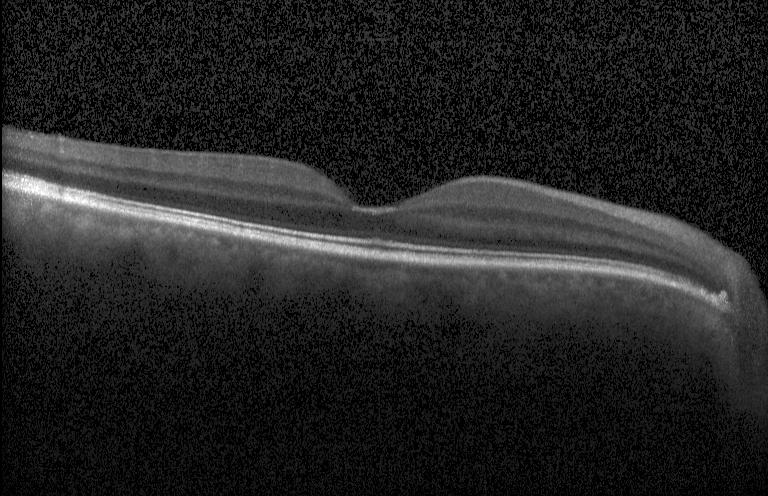

Macular OCT: neither choroidal neovascularization, diabetic macular edema, nor drusen.